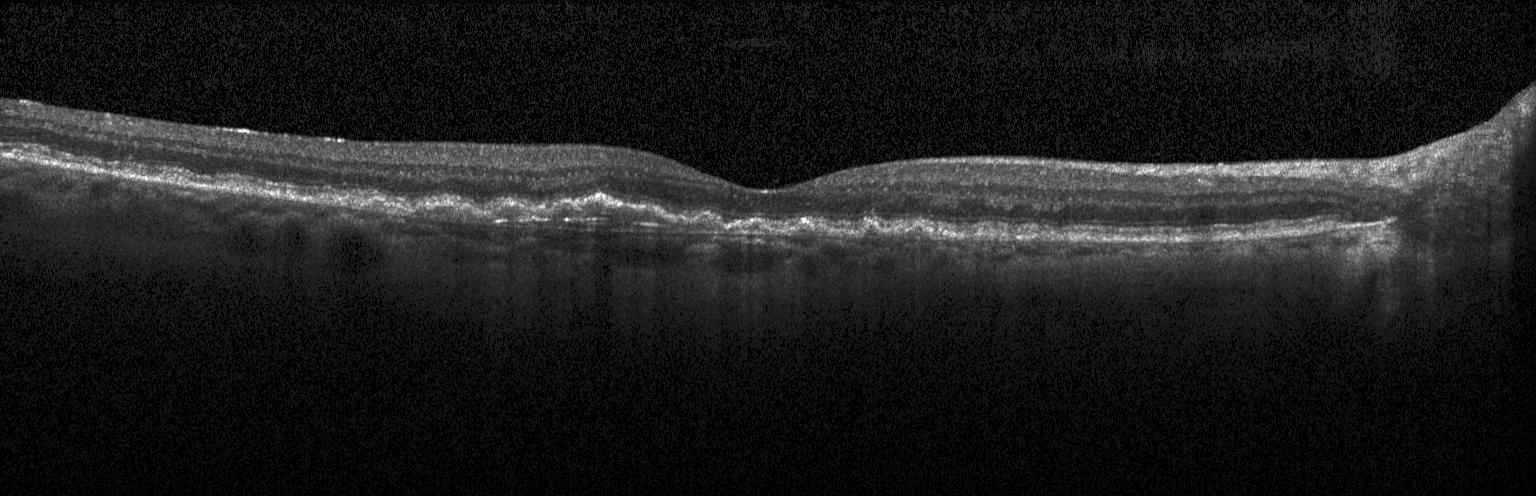
Retinal OCT B-scan. Diagnosis: choroidal neovascularization.